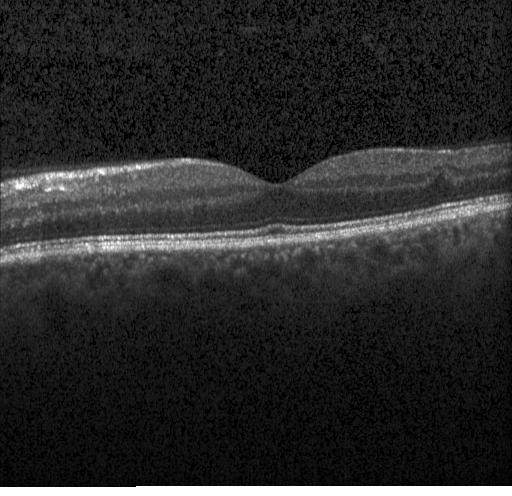 Retinal OCT B-scan; SD-OCT — Impression: no evidence of choroidal neovascularization, diabetic macular edema, or drusen.